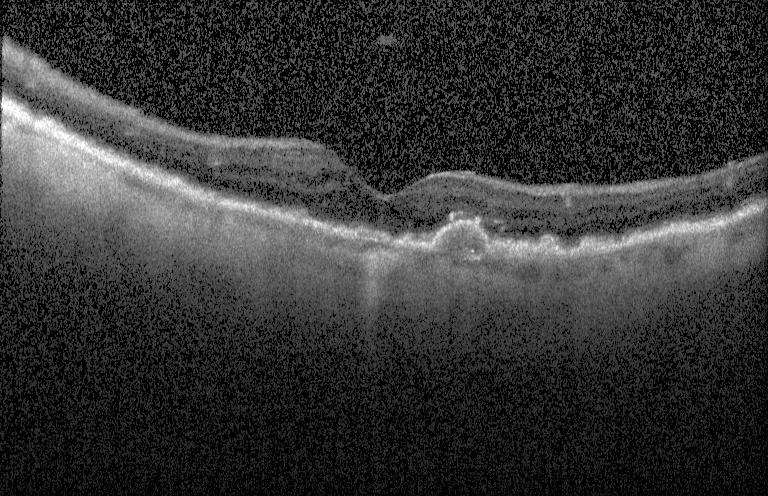 Spectral-domain OCT B-scan: a choroidal neovascular membrane.